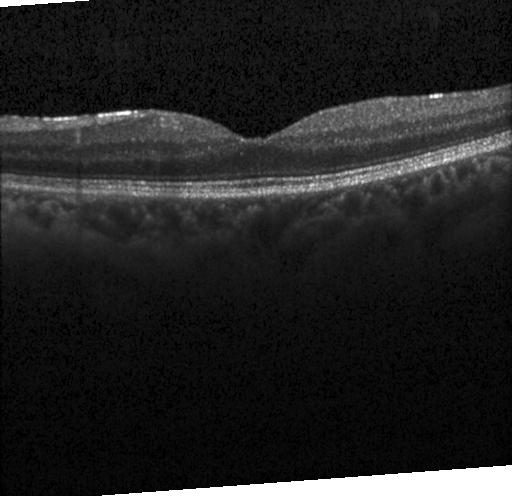

Spectral-domain OCT · retinal OCT B-scan.
Impression: no choroidal neovascularization, diabetic macular edema, or drusen.